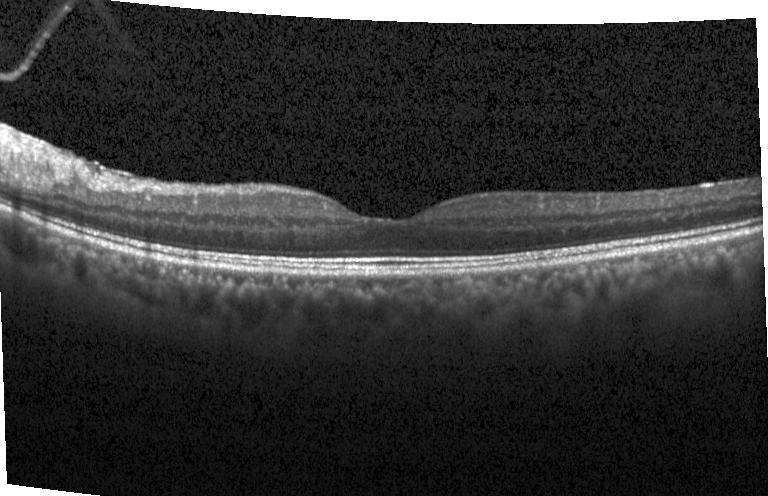

OCT B-scan showing neither choroidal neovascularization, diabetic macular edema, nor drusen.